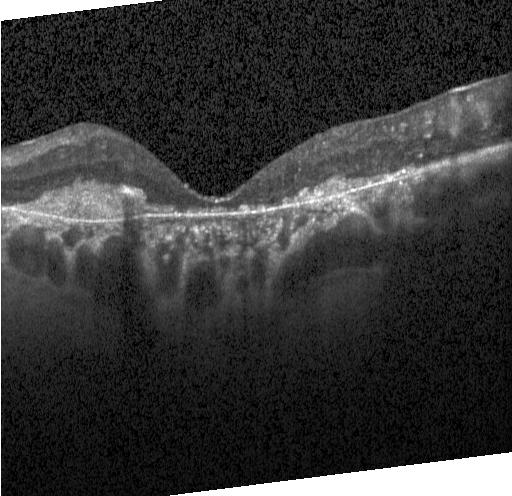

Spectral-domain OCT; optical coherence tomography B-scan; through the macula. Impression: choroidal neovascularization (CNV).